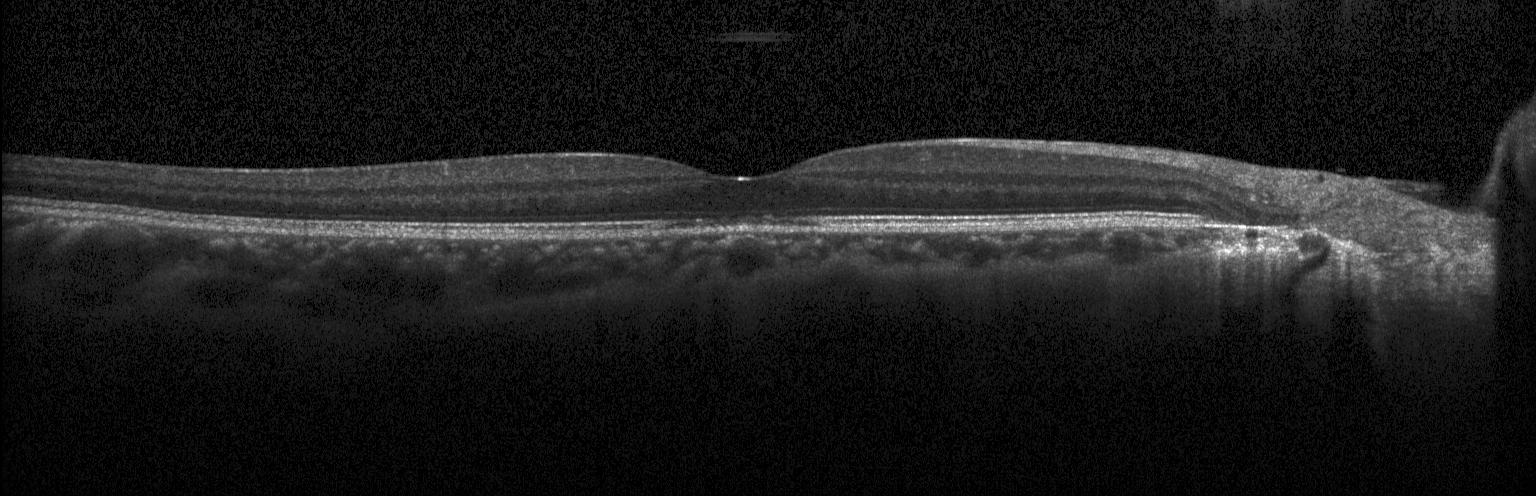

Finding: no evidence of choroidal neovascularization, diabetic macular edema, or drusen.